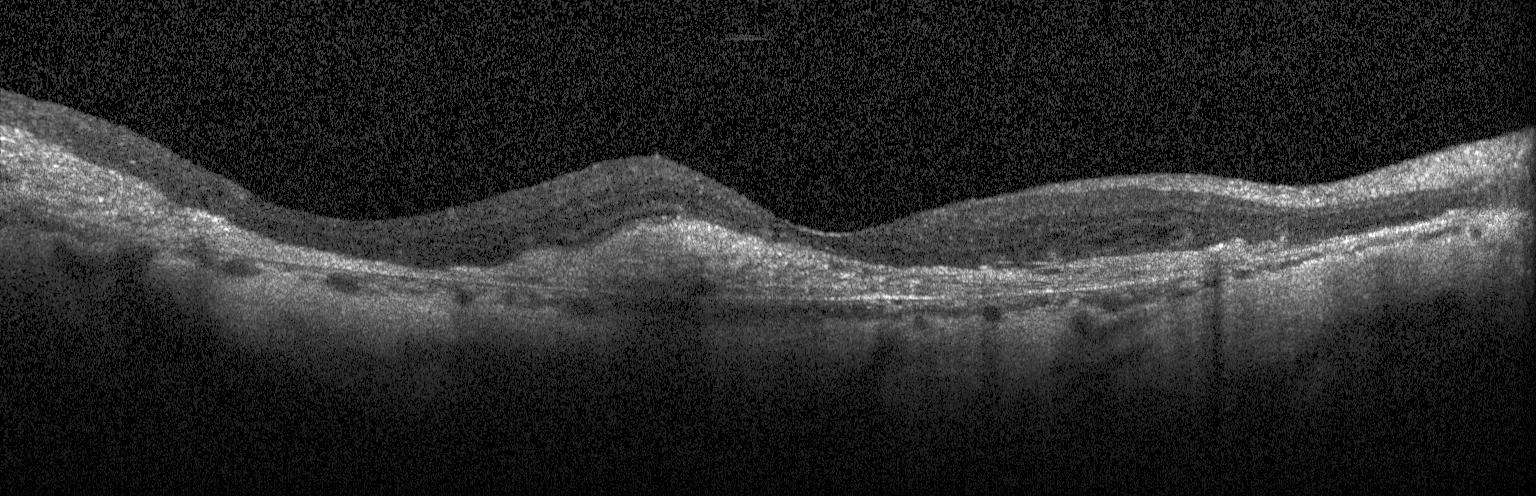

Heidelberg Spectralis OCT system; optical coherence tomography scan; horizontal scan through the fovea
Finding: choroidal neovascularization (CNV).